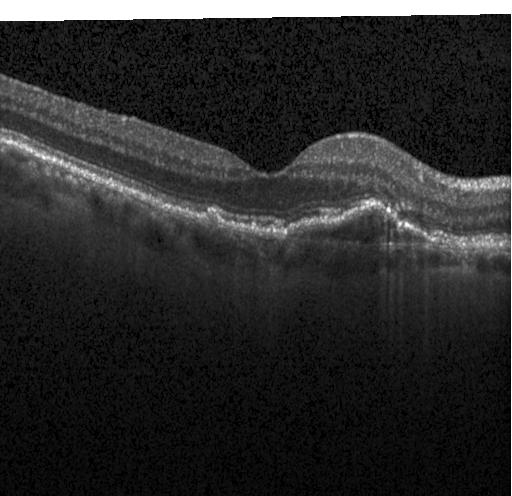
The scan shows a choroidal neovascular membrane.